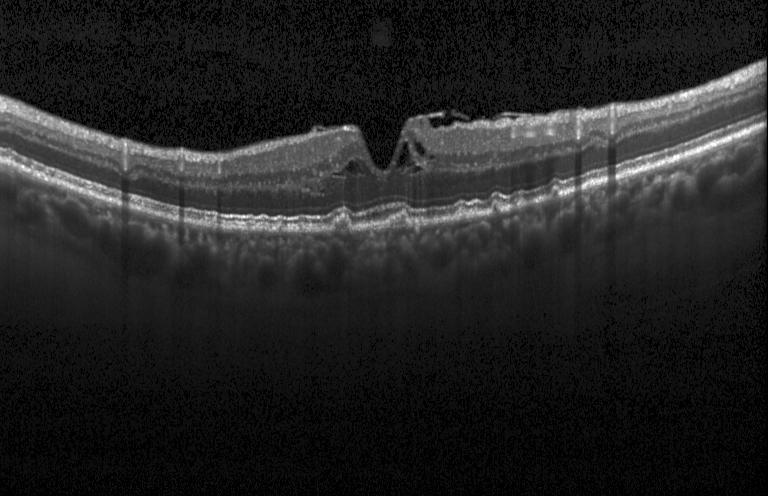

Assessment: drusen.